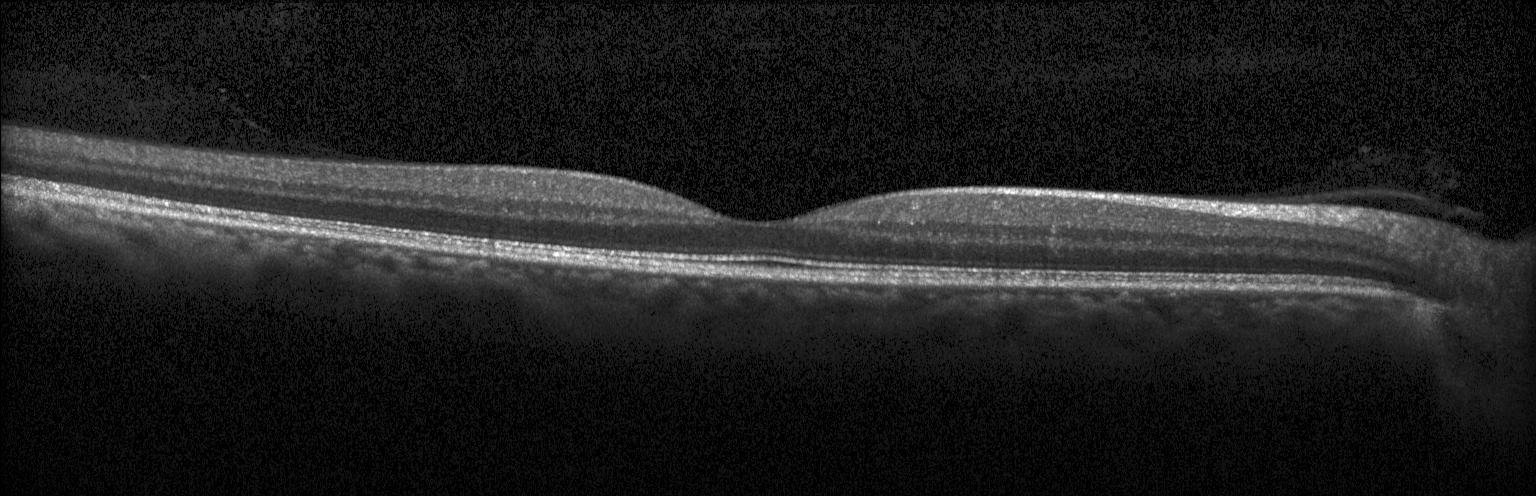 This B-scan demonstrates no evidence of choroidal neovascularization, diabetic macular edema, or drusen.